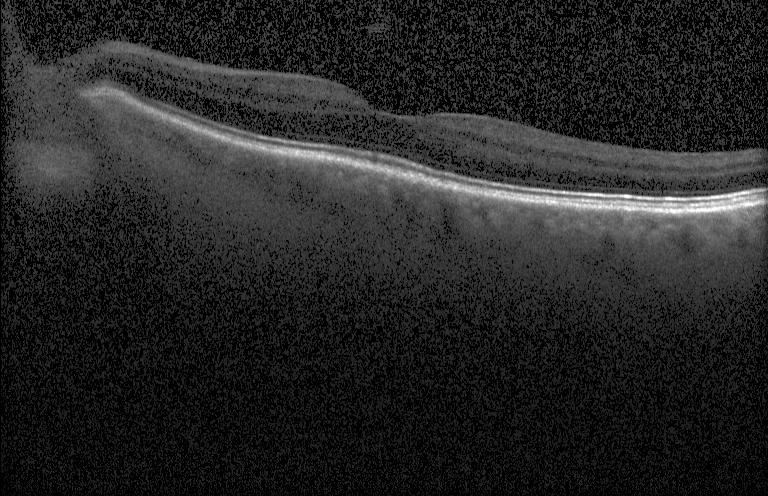
Spectral-domain OCT B-scan: no choroidal neovascularization, diabetic macular edema, or drusen.